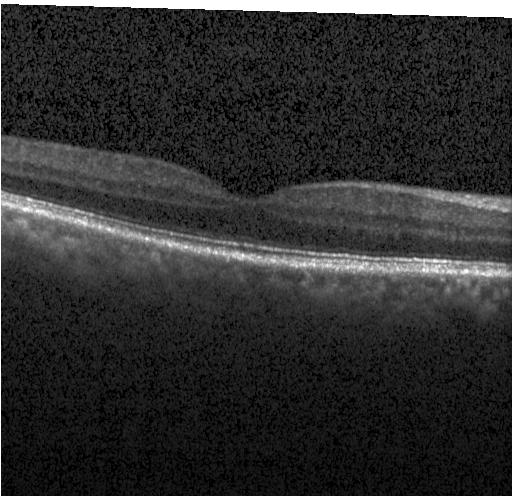 Spectral-domain OCT; instrument: Heidelberg Spectralis; optical coherence tomography scan; fovea-centered — The scan shows no choroidal neovascularization, no diabetic macular edema, and no drusen.